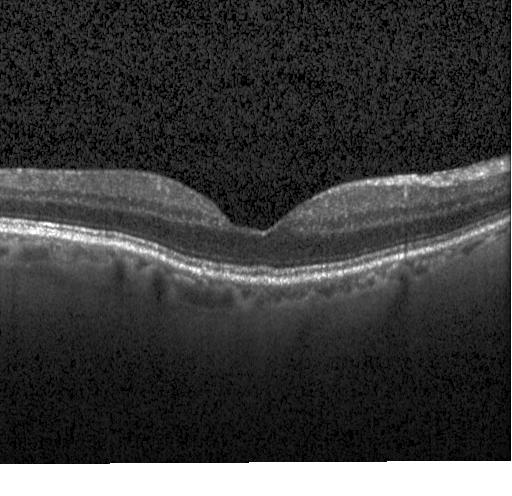 Diagnosis: no CNV, DME, or drusen.